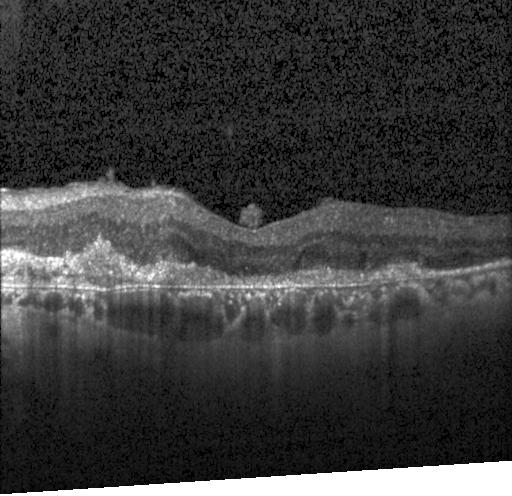

Macular OCT demonstrating CNV.